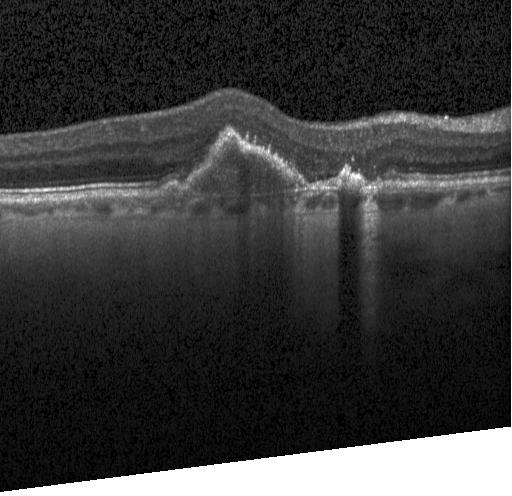

The scan shows choroidal neovascularization (CNV).